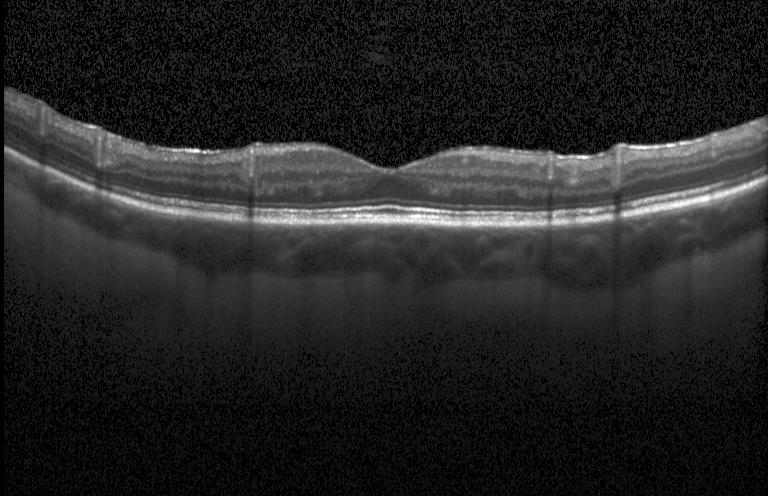

Dx: no evidence of choroidal neovascularization, diabetic macular edema, or drusen.